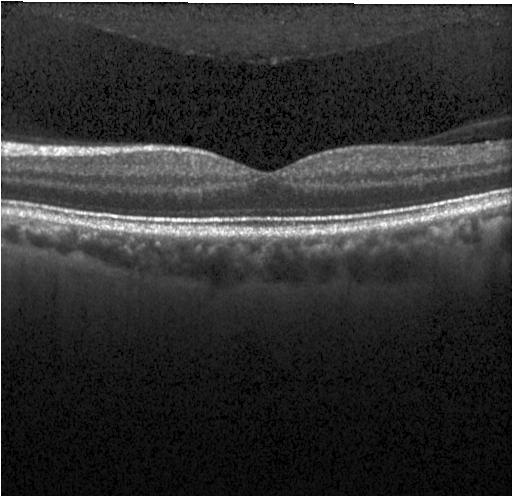
Optical coherence tomography scan; Heidelberg Spectralis; SD-OCT. OCT finding: no CNV, DME, or drusen.